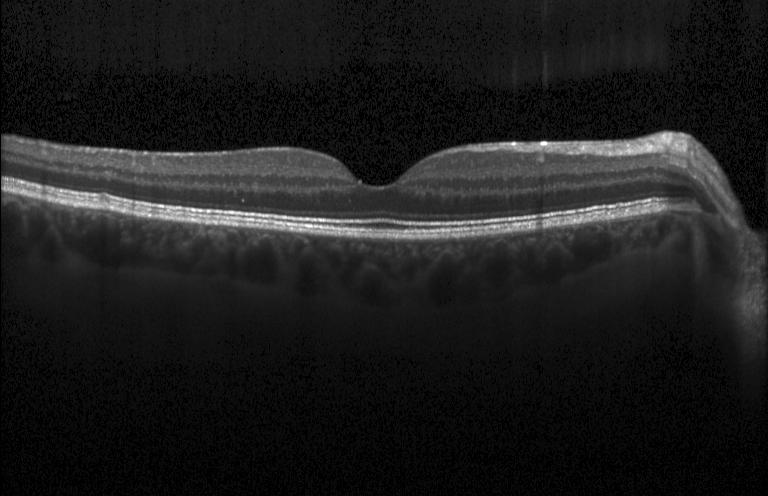
Retinal OCT cross-section · acquired on a Heidelberg Spectralis.
Macular OCT: no evidence of CNV, DME, or drusen.